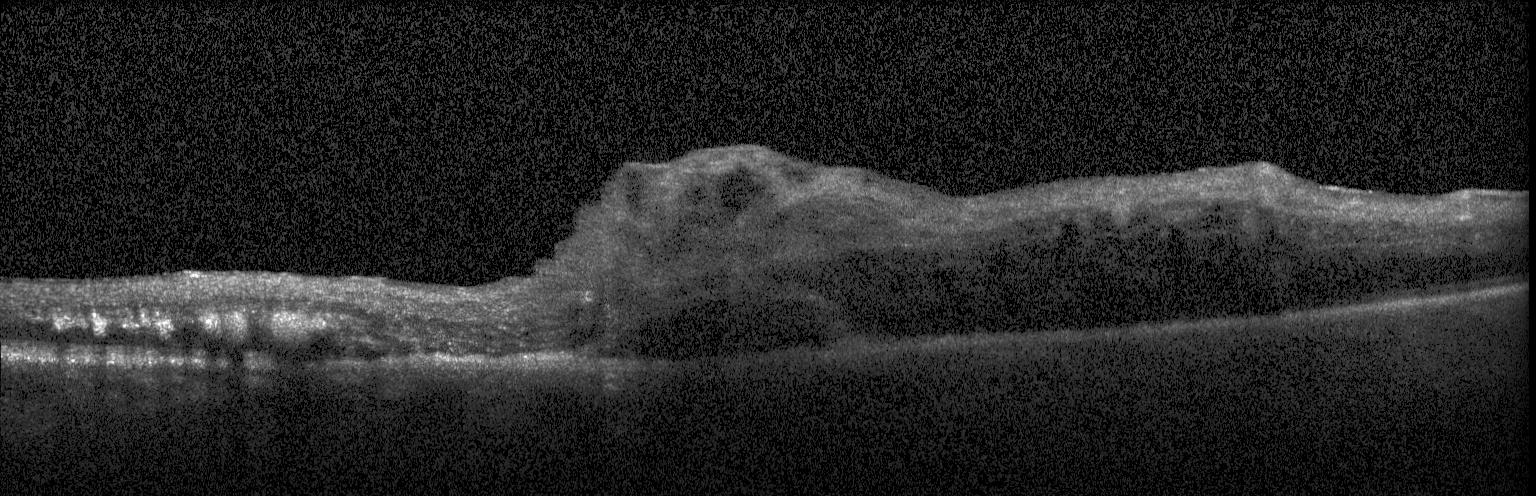
Macular OCT demonstrating CNV.